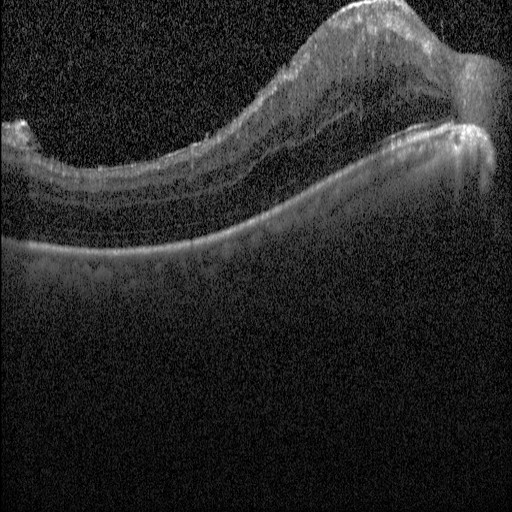 OCT line scan
Macular OCT: diabetic macular edema (DME).